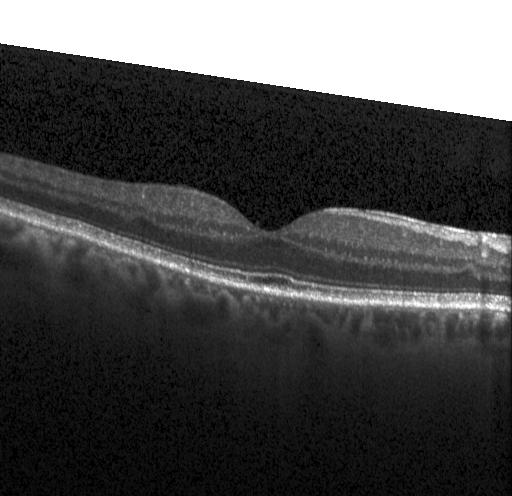 Heidelberg Spectralis, retinal OCT cross-section, centered on the fovea. Diagnosis: no choroidal neovascularization, diabetic macular edema, or drusen.